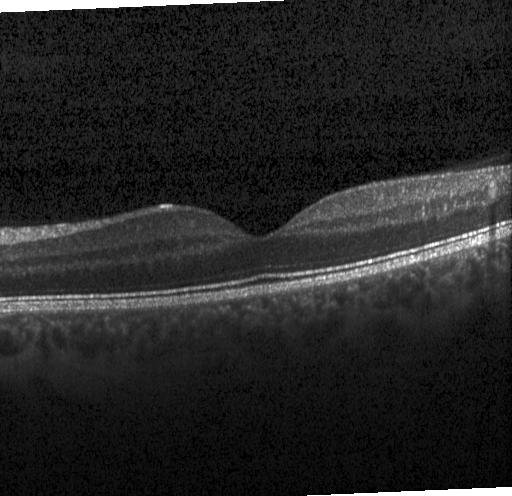 Centered on the fovea, OCT line scan.
Finding: no choroidal neovascularization, diabetic macular edema, or drusen.